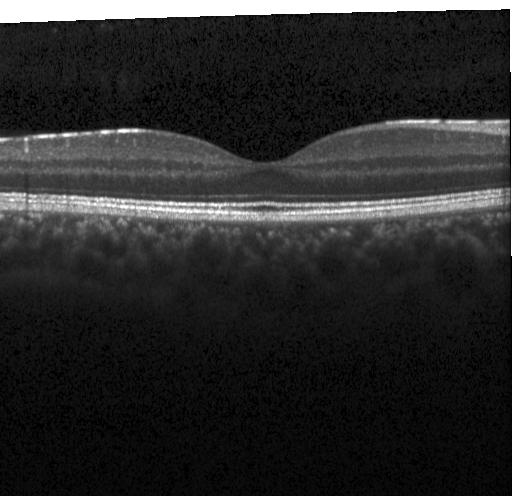
Spectral-domain OCT B-scan: neither CNV, DME, nor drusen.